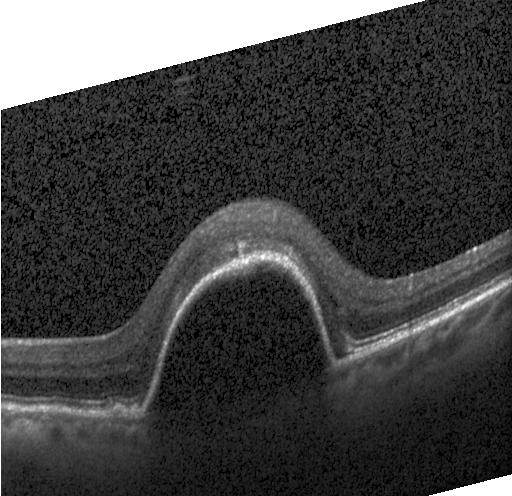
OCT scan showing choroidal neovascularization.